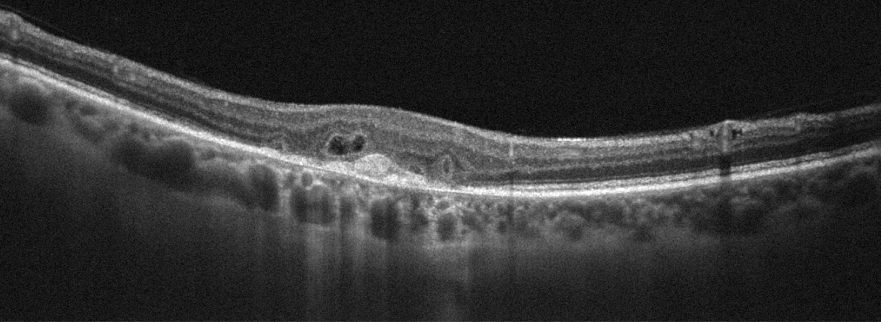 The scan shows AMD.